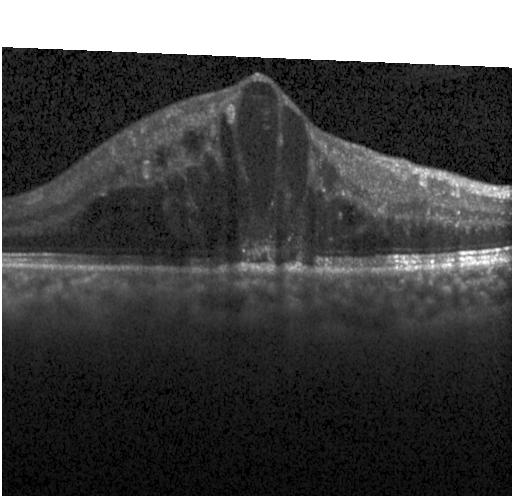 Macular OCT demonstrating diabetic macular edema (DME).